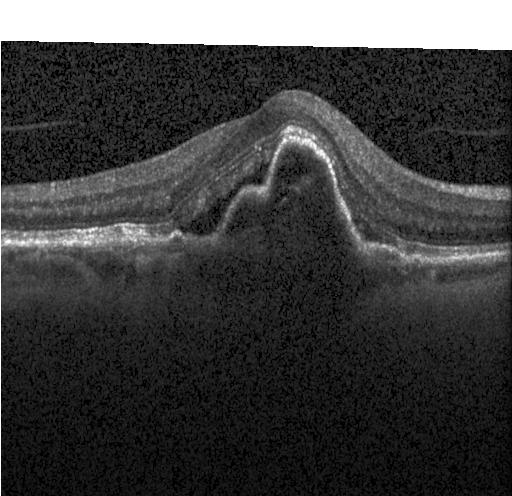

Instrument: Heidelberg Spectralis. Retinal OCT B-scan. Choroidal neovascularization.